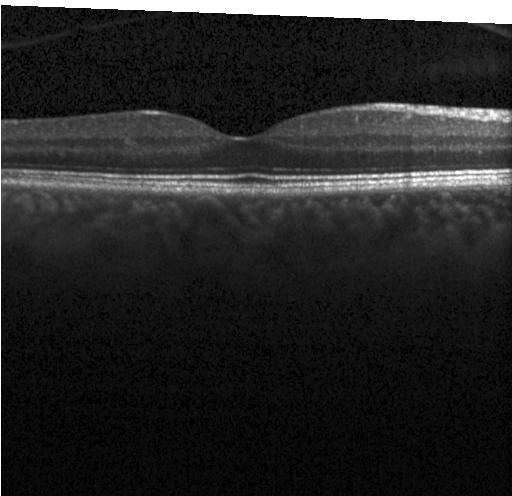
Heidelberg Spectralis; spectral-domain optical coherence tomography; optical coherence tomography scan — Assessment: no choroidal neovascularization, no diabetic macular edema, and no drusen.